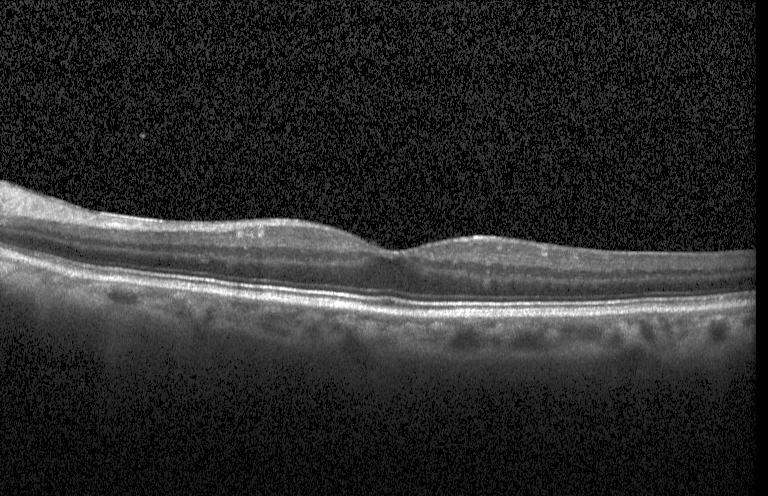

Macular OCT demonstrating no evidence of choroidal neovascularization, diabetic macular edema, or drusen.